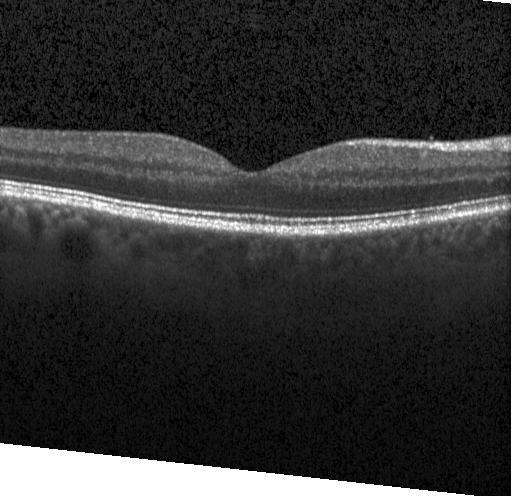
Centered on the fovea · OCT line scan · spectral-domain optical coherence tomography.
Finding: no choroidal neovascularization, no diabetic macular edema, and no drusen.